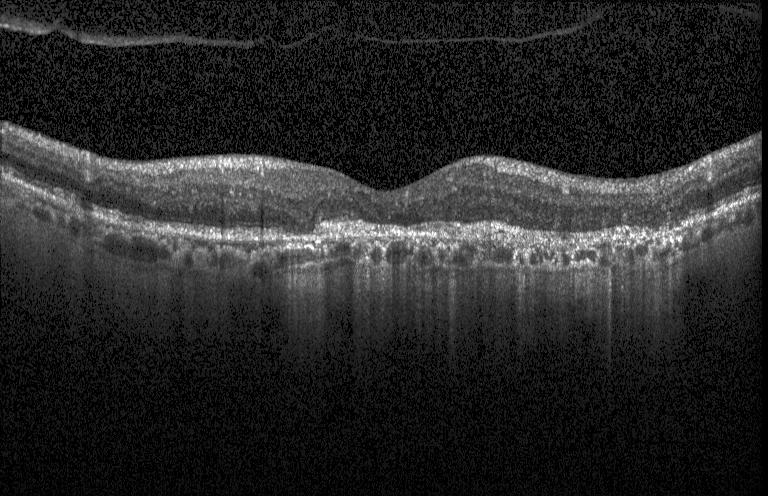
Finding: a choroidal neovascular membrane.